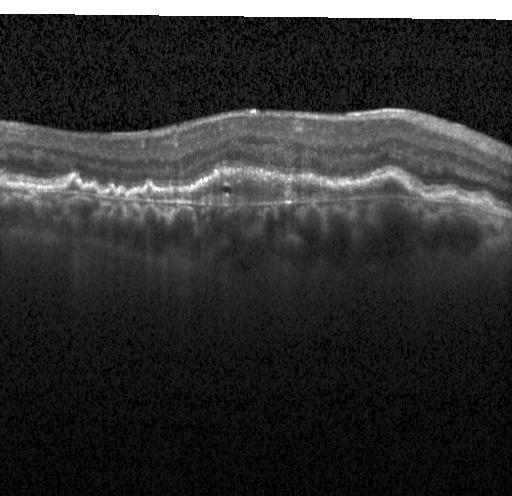

Optical coherence tomography scan · horizontal scan through the fovea · acquired on a Heidelberg Spectralis · SD-OCT — OCT finding: choroidal neovascularization (CNV).